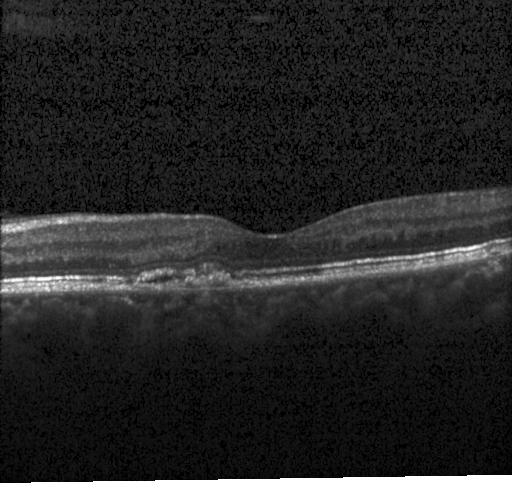

Assessment: a choroidal neovascular membrane.